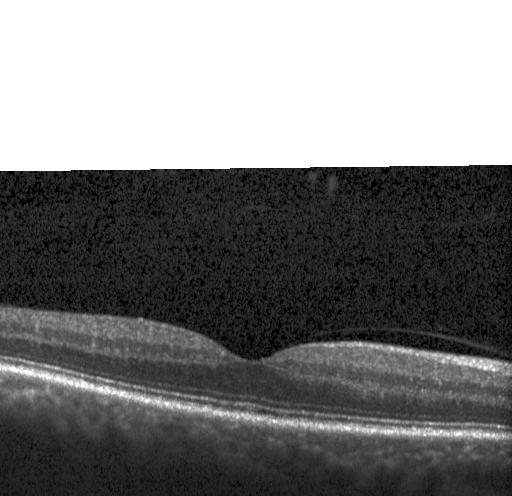 Finding: no evidence of choroidal neovascularization, diabetic macular edema, or drusen.